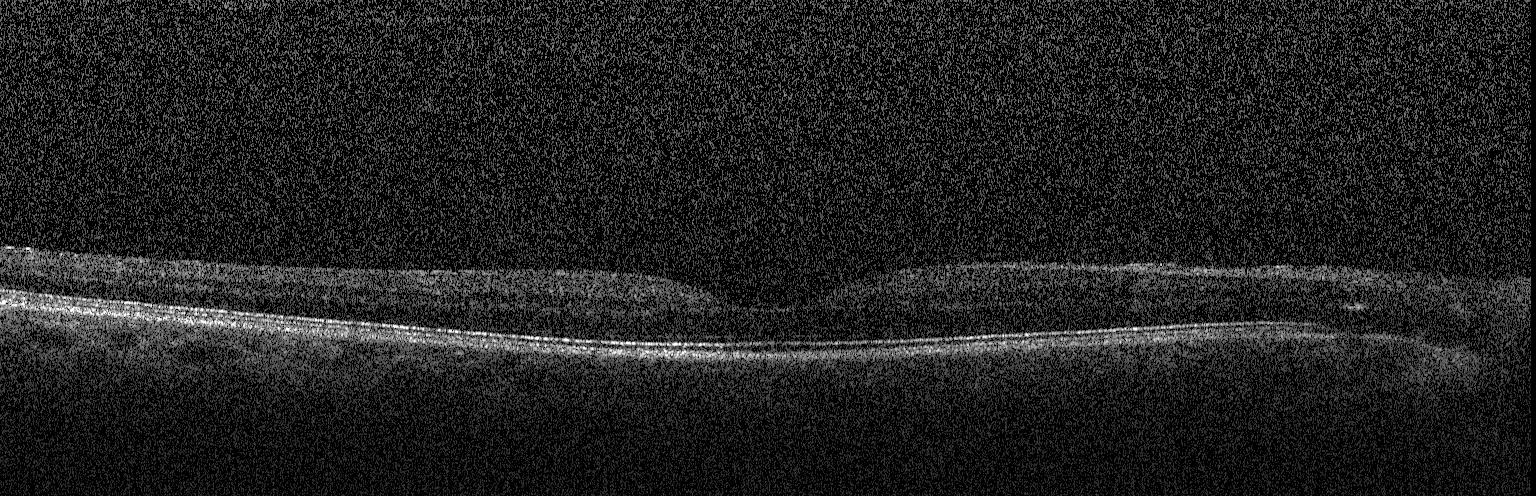

Finding: no CNV, no DME, and no drusen.